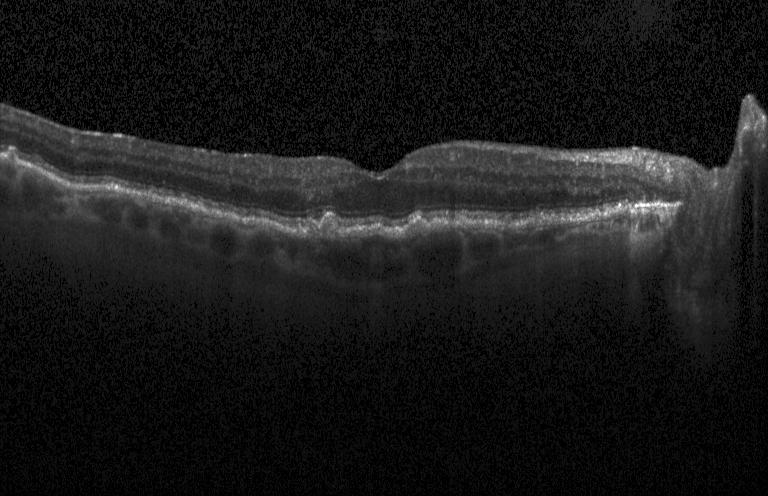

Optical coherence tomography scan, macular scan, spectral-domain OCT, instrument: Heidelberg Spectralis. Assessment: drusen.